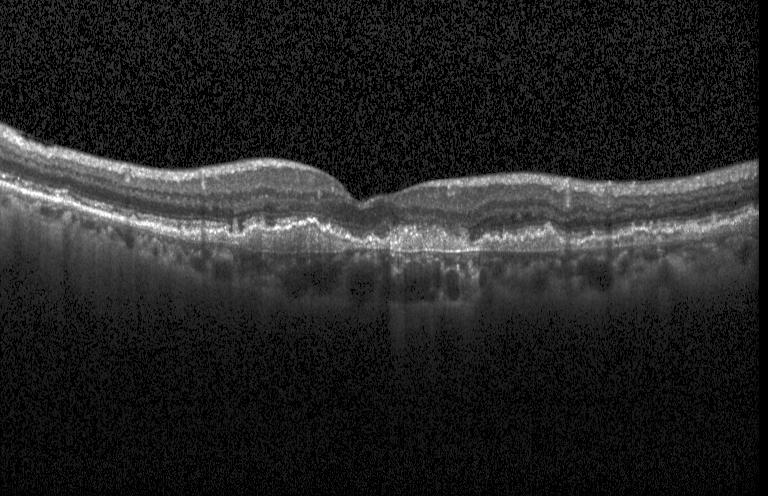

OCT B-scan, SD-OCT, instrument: Heidelberg Spectralis
Diagnosis: choroidal neovascularization (CNV).